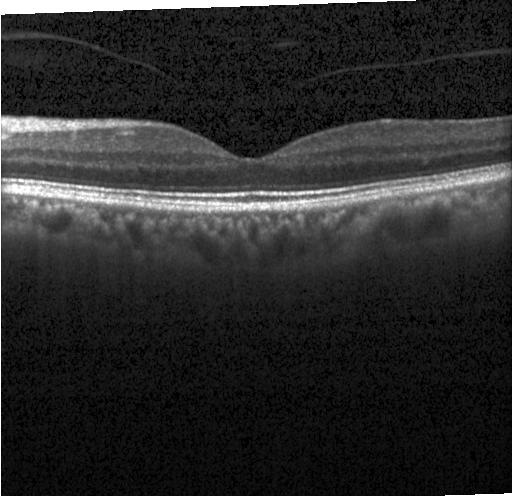
OCT B-scan. Diagnosis: no choroidal neovascularization, diabetic macular edema, or drusen.